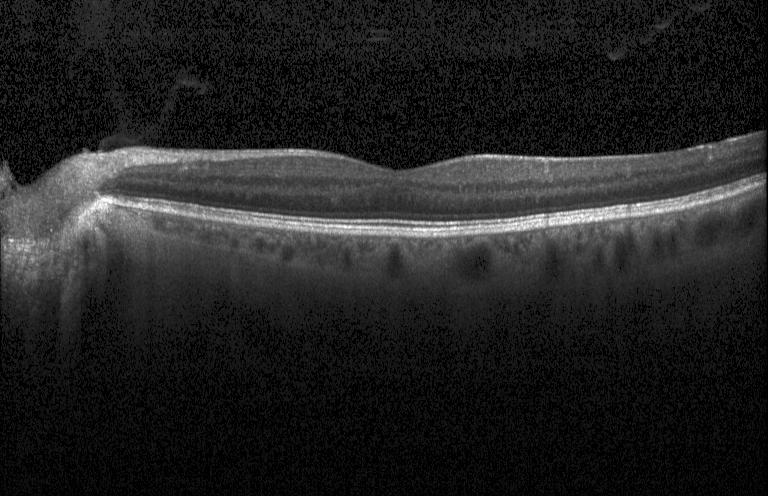

Optical coherence tomography scan. Centered on the fovea
Impression: no choroidal neovascularization, diabetic macular edema, or drusen.